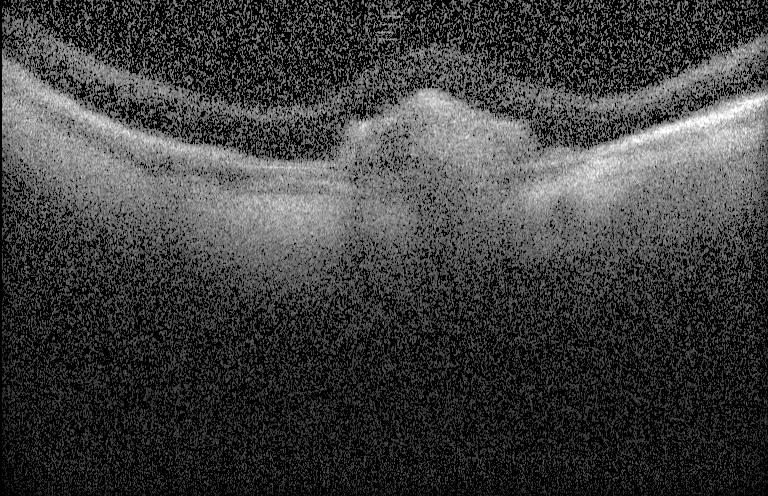

Impression: a choroidal neovascular membrane.